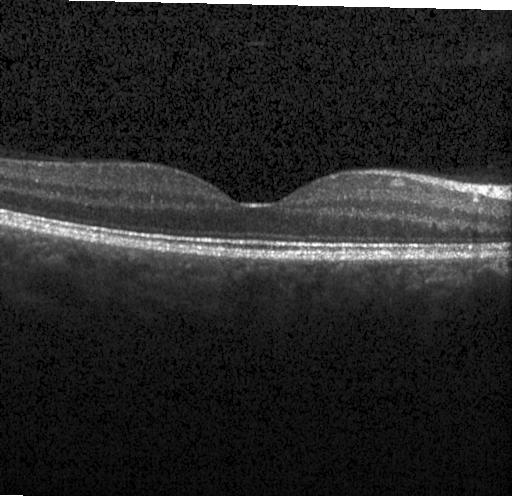 Spectral-domain OCT, acquired on a Heidelberg Spectralis, horizontal scan through the fovea, optical coherence tomography scan.
Finding: neither CNV, DME, nor drusen.